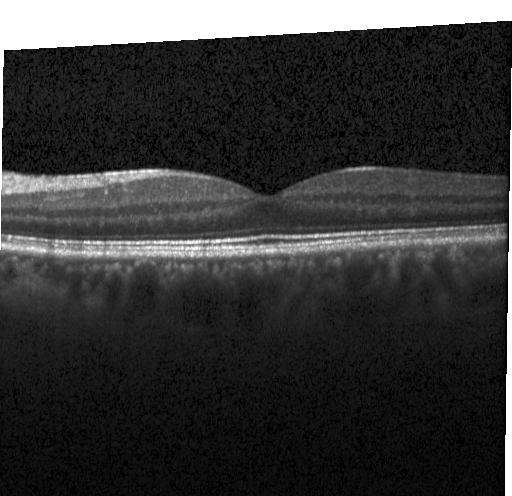 Spectral-domain optical coherence tomography; retinal OCT B-scan
The scan shows neither CNV, DME, nor drusen.